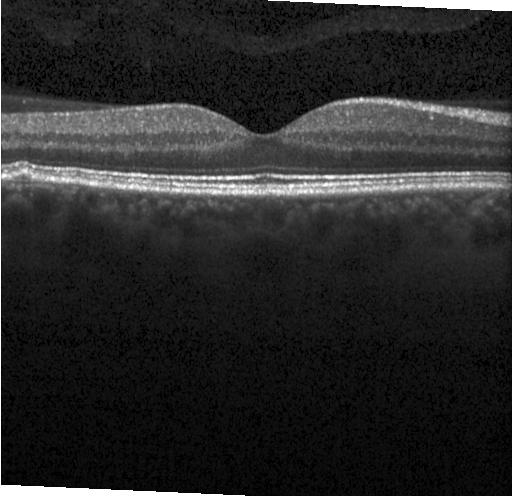

Optical coherence tomography scan. Spectral-domain optical coherence tomography. Heidelberg Spectralis OCT system. The scan shows drusen.